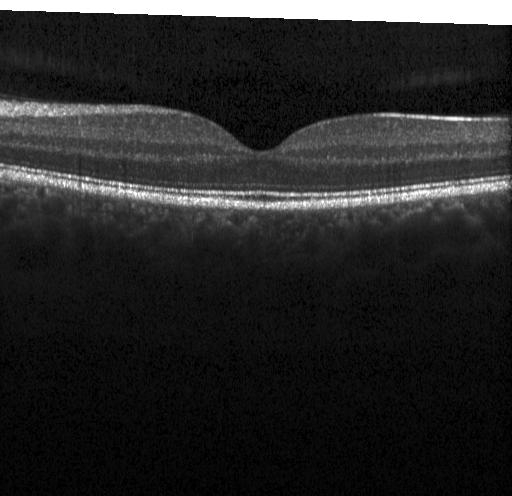

Spectral-domain OCT. Retinal OCT cross-section. Horizontal scan through the fovea — Finding: neither choroidal neovascularization, diabetic macular edema, nor drusen.